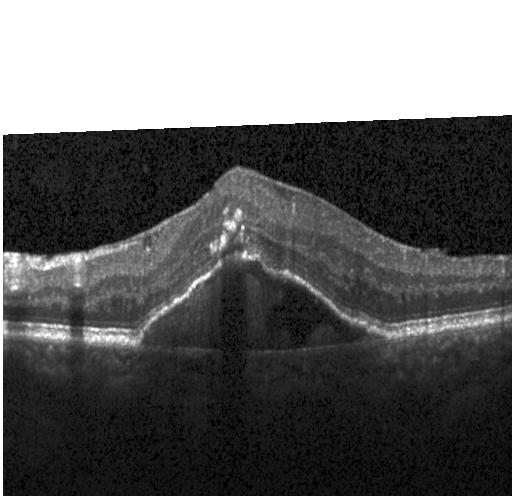 Through the macula. Acquired on a Heidelberg Spectralis. Optical coherence tomography scan. Spectral-domain optical coherence tomography. Diagnosis: a choroidal neovascular membrane.